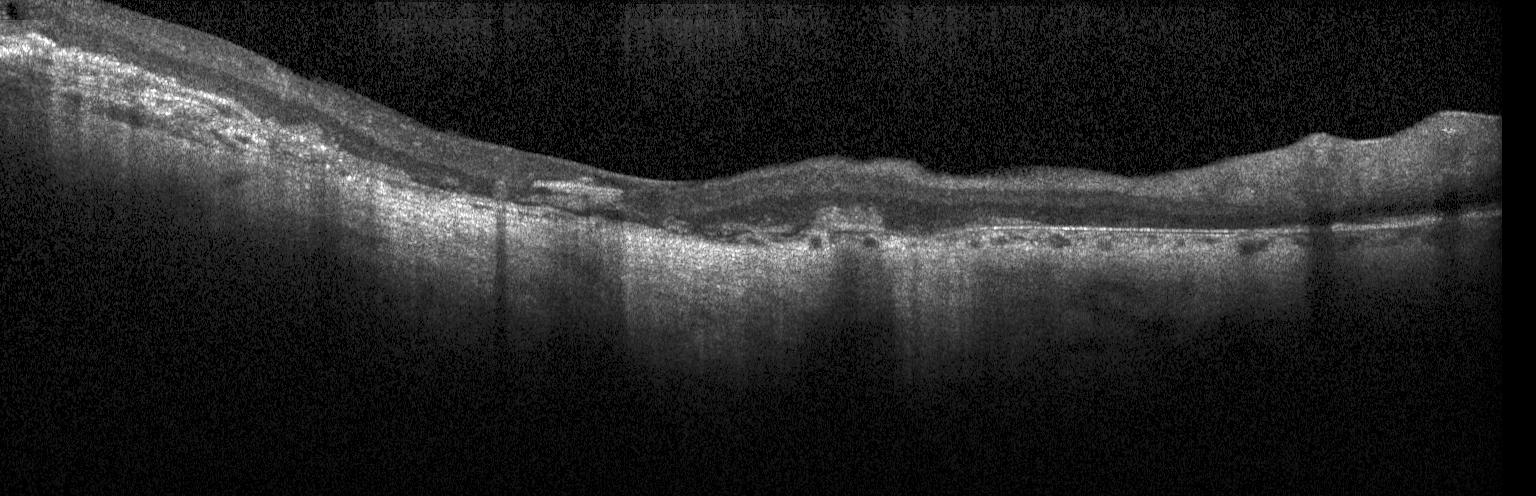
Retinal OCT cross-section. Macular OCT: CNV.